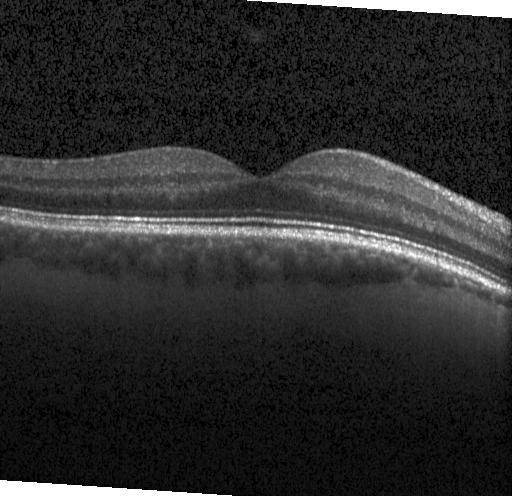

Heidelberg Spectralis OCT system, optical coherence tomography scan, SD-OCT. No choroidal neovascularization, no diabetic macular edema, and no drusen.